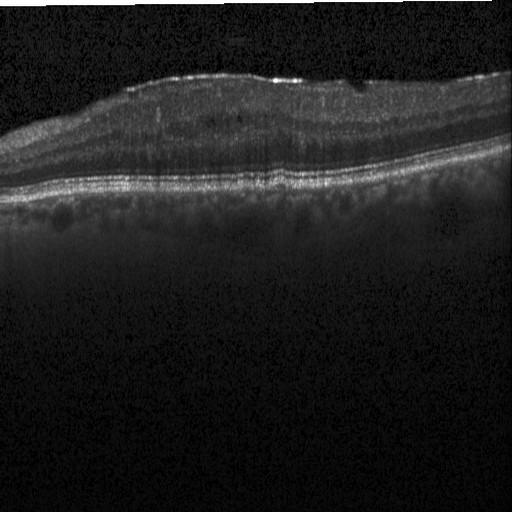 Impression: diabetic macular edema (DME).